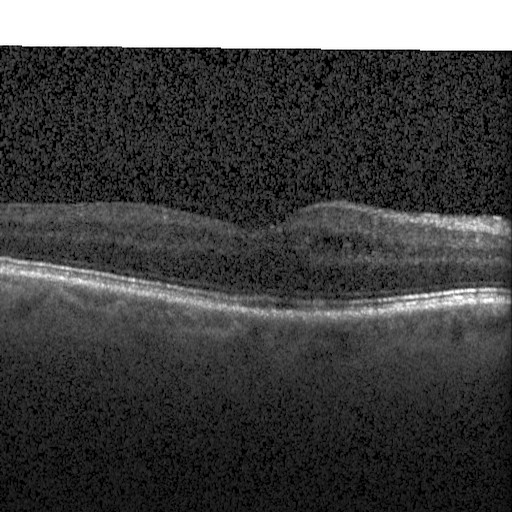

Macular scan; OCT line scan; spectral-domain optical coherence tomography — Diagnosis: DME.